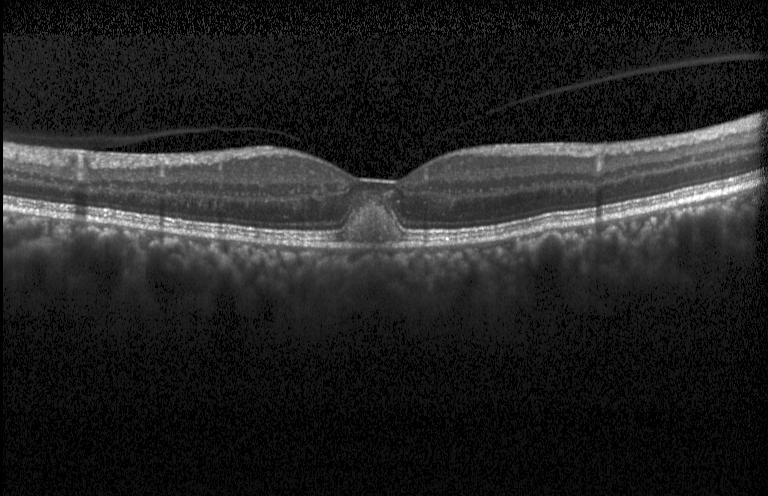

Optical coherence tomography B-scan.
Macular OCT: a choroidal neovascular membrane.